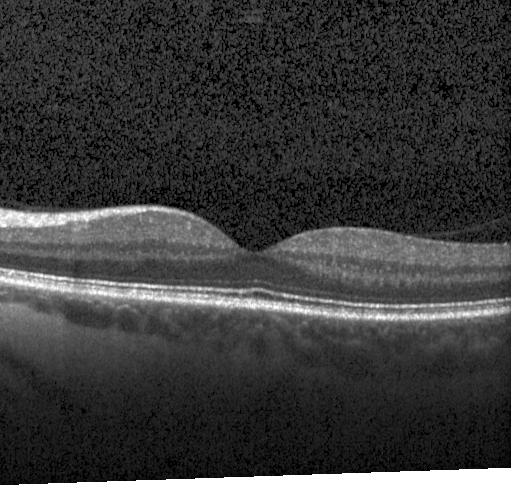 Optical coherence tomography B-scan — Impression: no evidence of choroidal neovascularization, diabetic macular edema, or drusen.